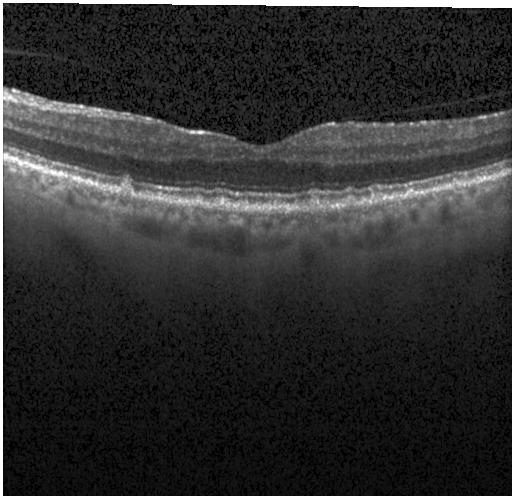 Spectral-domain OCT. OCT line scan.
Macular OCT: drusen.